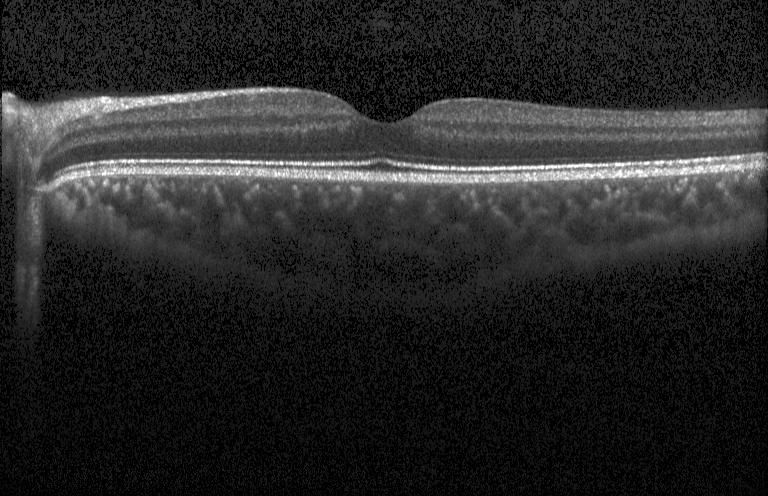

Retinal OCT cross-section. Diagnosis: no choroidal neovascularization, diabetic macular edema, or drusen.